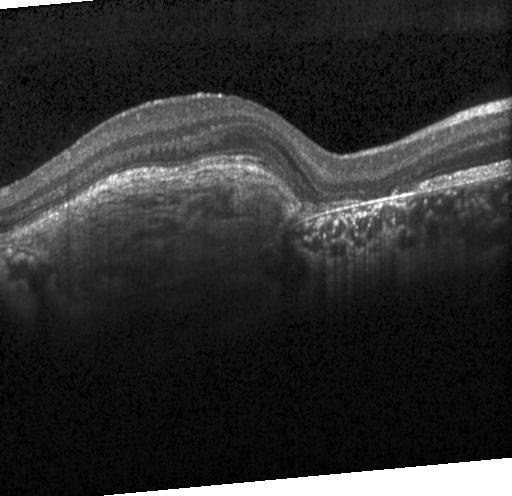 OCT scan showing a choroidal neovascular membrane.